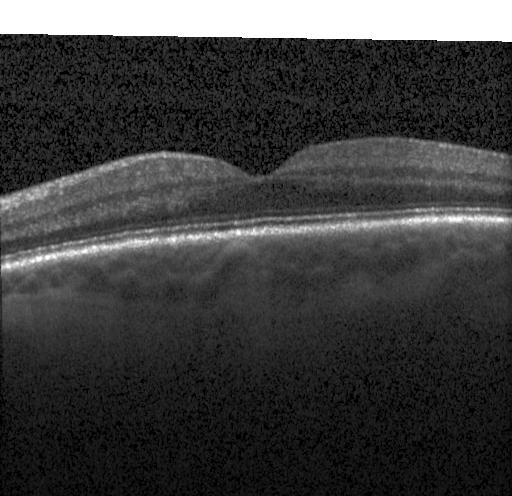
The scan shows no CNV, DME, or drusen.